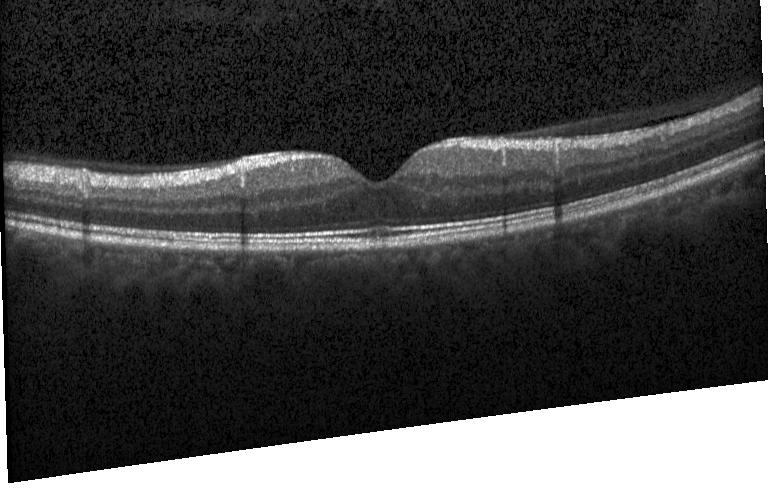

Retinal OCT cross-section.
Impression: neither choroidal neovascularization, diabetic macular edema, nor drusen.